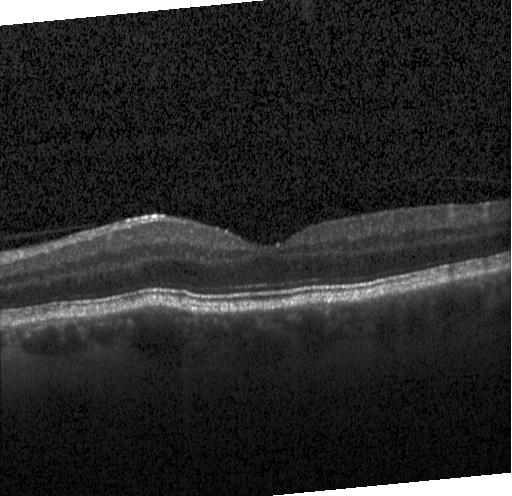
Impression: no CNV, no DME, and no drusen.